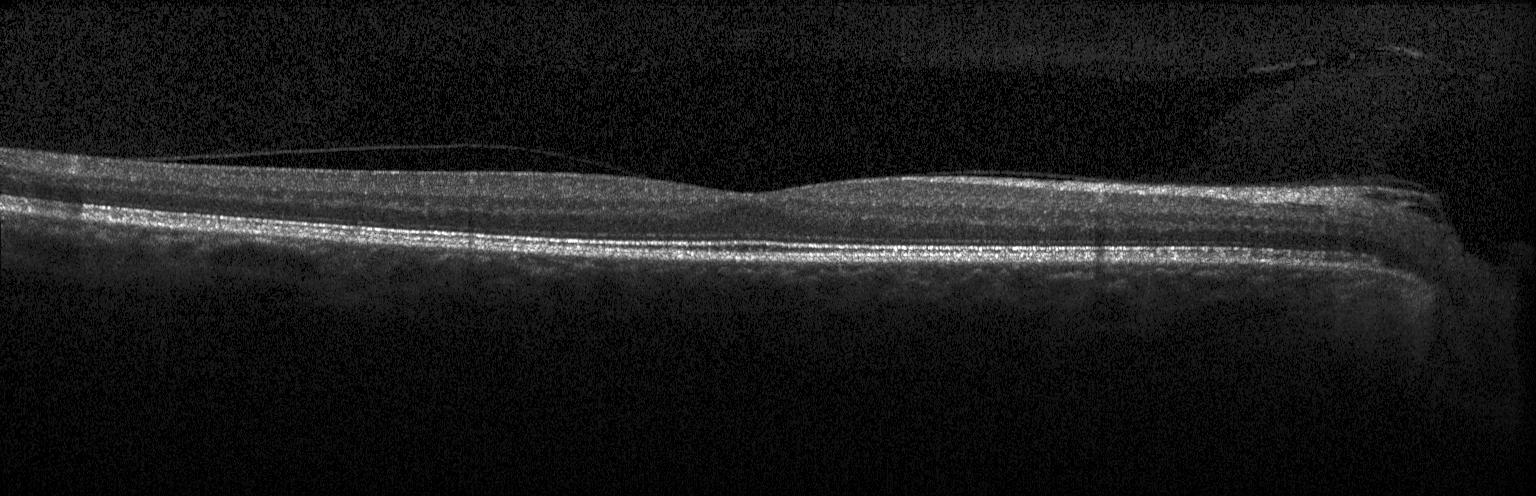
Heidelberg Spectralis OCT system. Optical coherence tomography B-scan — Impression: neither choroidal neovascularization, diabetic macular edema, nor drusen.